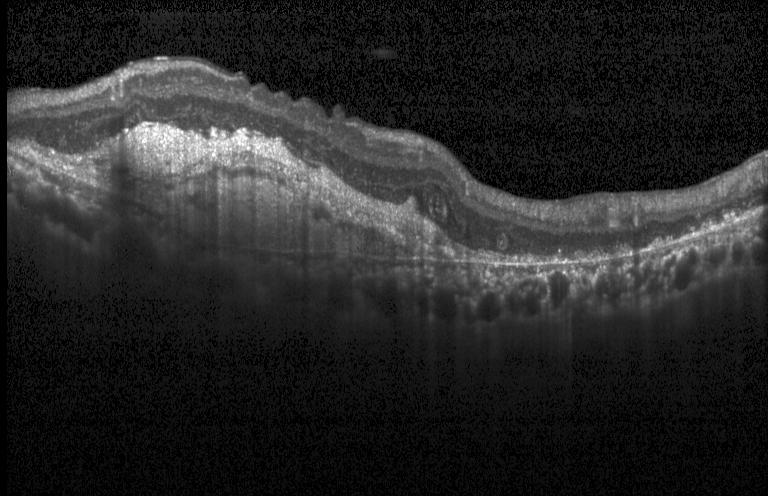 OCT line scan. Fovea-centered. Acquired on a Heidelberg Spectralis. SD-OCT.
The scan shows CNV.